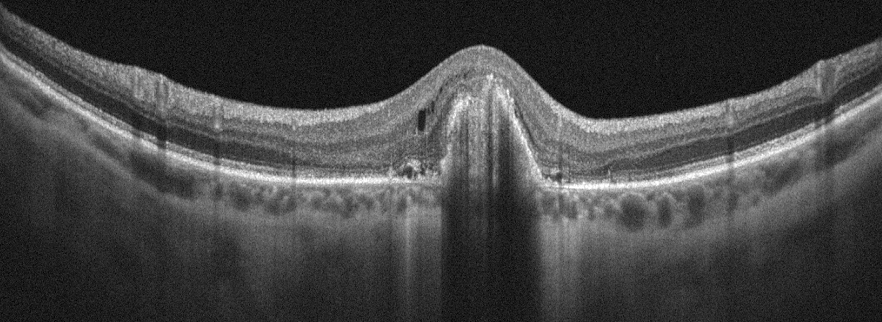
OD. Acquired on an Optovue Avanti RTVue XR. Retinal OCT B-scan. Fovea-centered.
Finding: age-related macular degeneration (AMD).